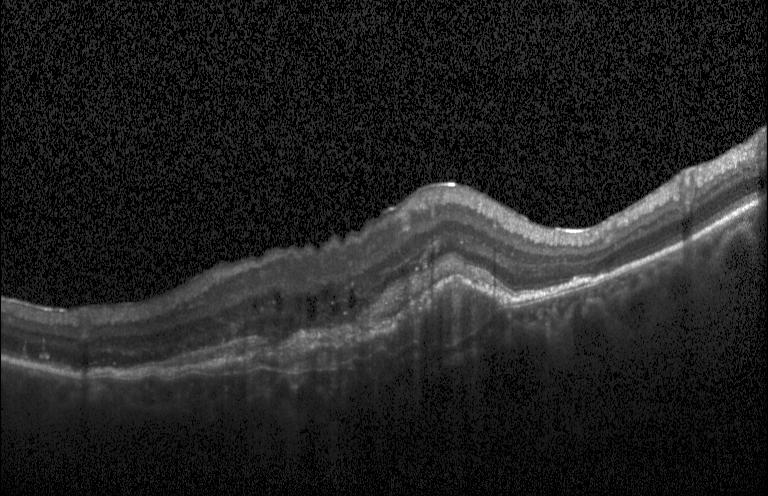
Spectral-domain optical coherence tomography · centered on the fovea · optical coherence tomography B-scan
Macular OCT: a choroidal neovascular membrane.